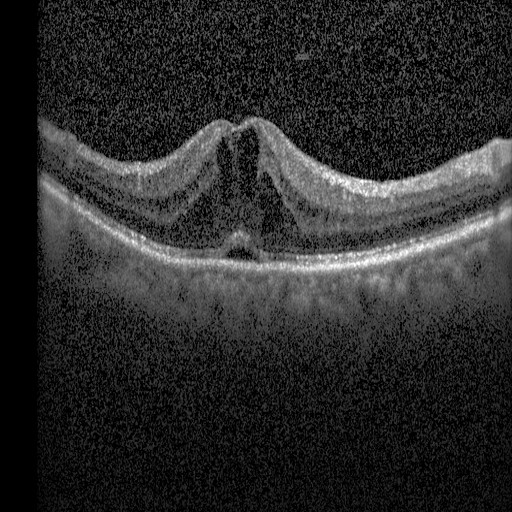

OCT scan showing diabetic macular edema.